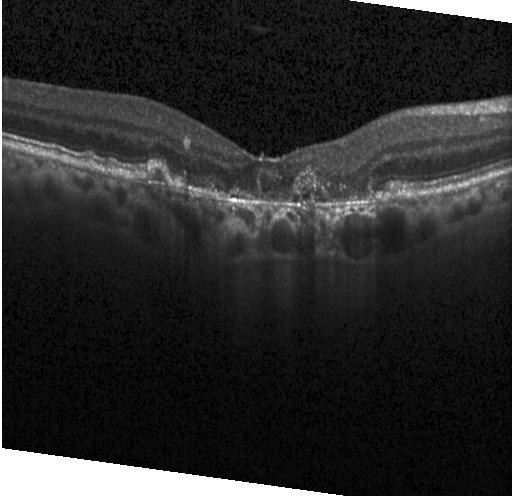 Centered on the fovea; spectral-domain OCT; optical coherence tomography scan — Finding: choroidal neovascularization.